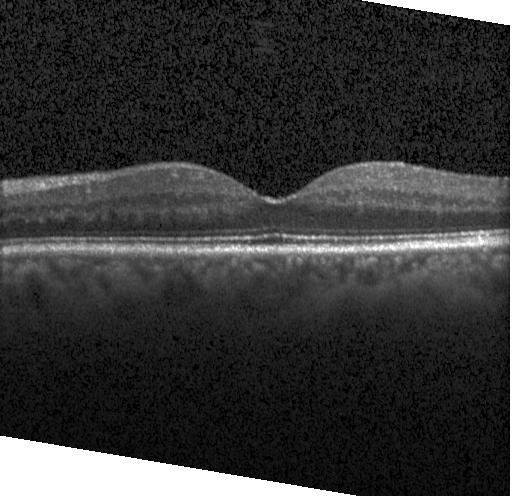
Instrument: Heidelberg Spectralis. OCT B-scan. SD-OCT.
Impression: no evidence of choroidal neovascularization, diabetic macular edema, or drusen.